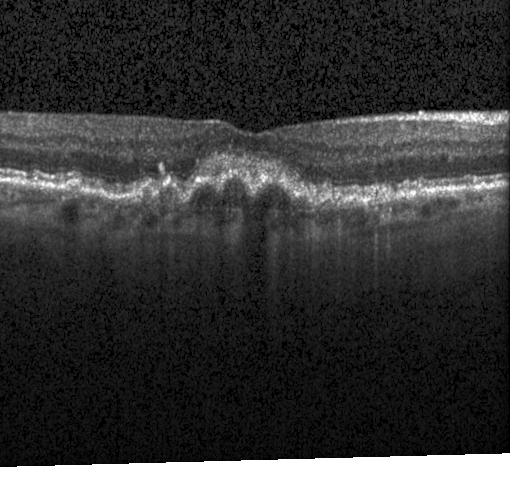

Instrument: Heidelberg Spectralis, optical coherence tomography scan
A choroidal neovascular membrane.